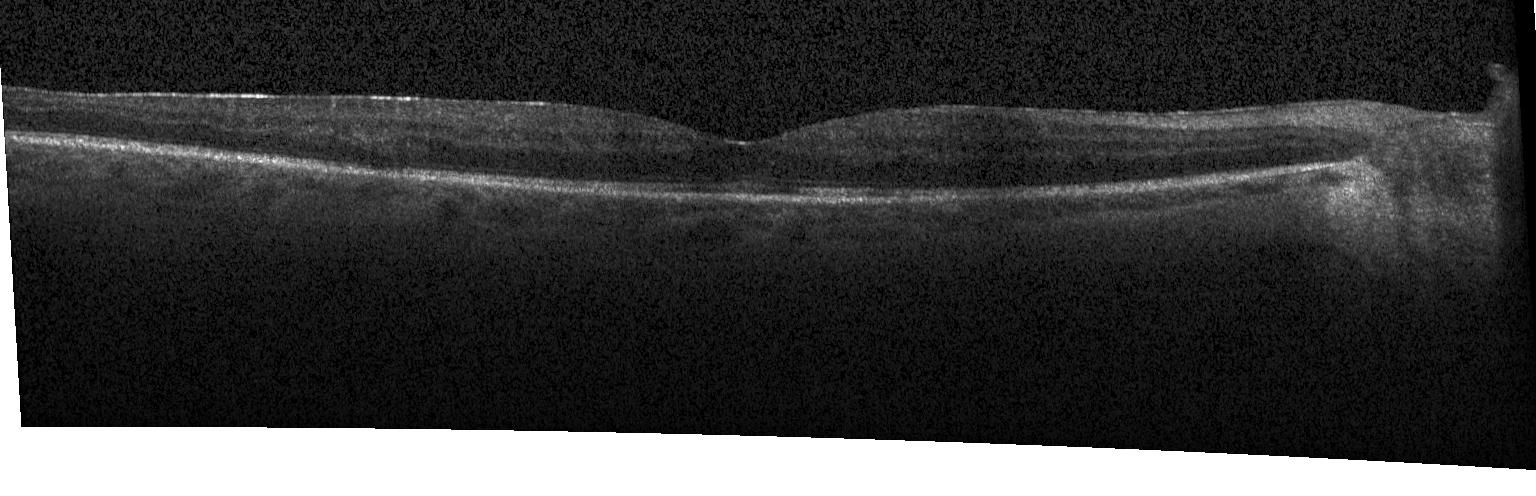 Assessment: no choroidal neovascularization, diabetic macular edema, or drusen.